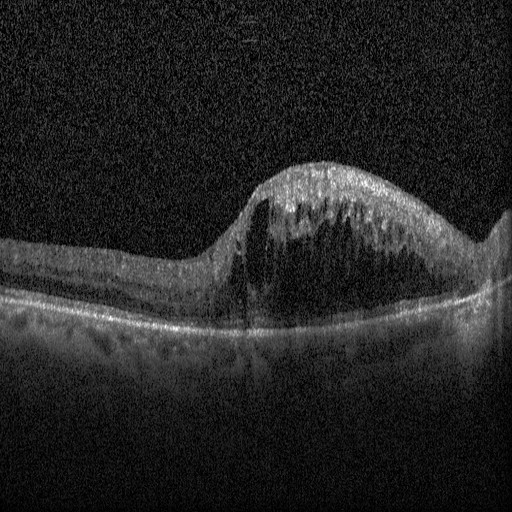 Through the macula. OCT line scan — The scan shows diabetic macular edema.